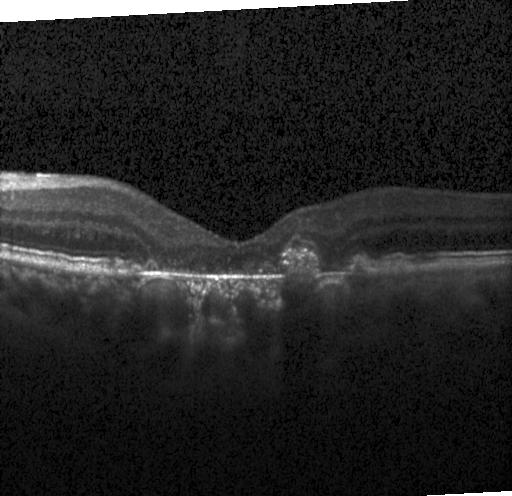

OCT scan showing a choroidal neovascular membrane.